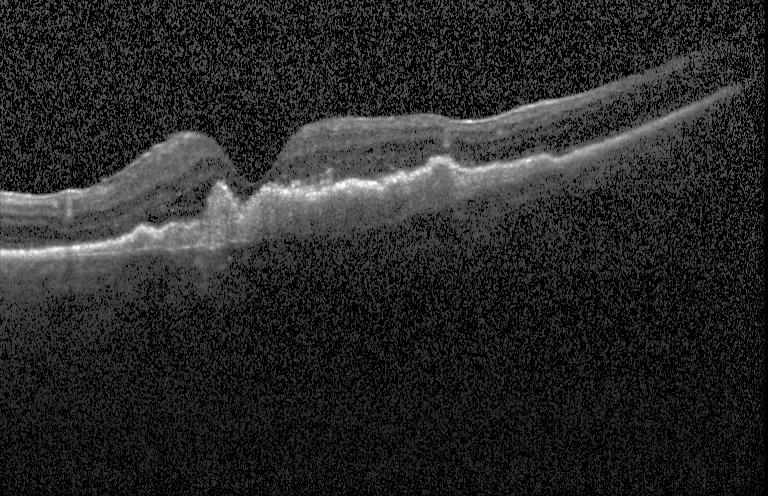 Heidelberg Spectralis · horizontal scan through the fovea · retinal OCT B-scan · spectral-domain OCT. The scan shows a choroidal neovascular membrane.